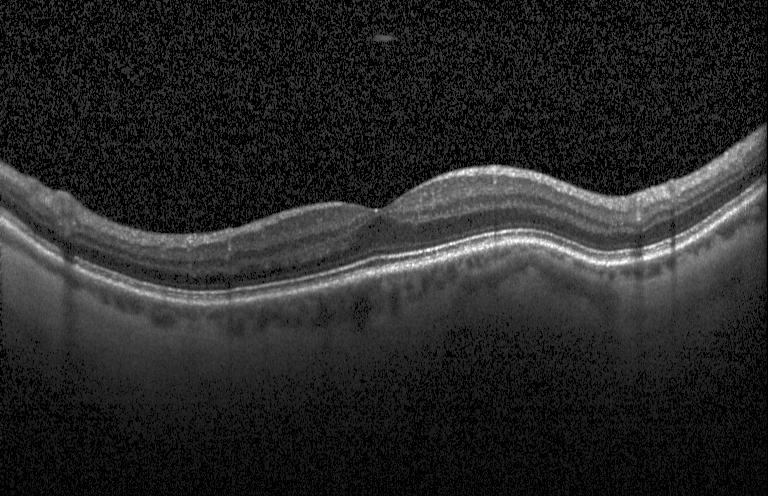

Macular OCT: no choroidal neovascularization, no diabetic macular edema, and no drusen.